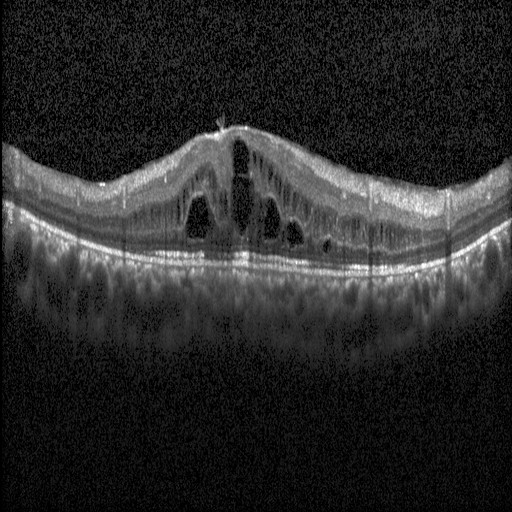
Heidelberg Spectralis OCT system · spectral-domain optical coherence tomography · through the macula · retinal OCT cross-section. This B-scan demonstrates DME.